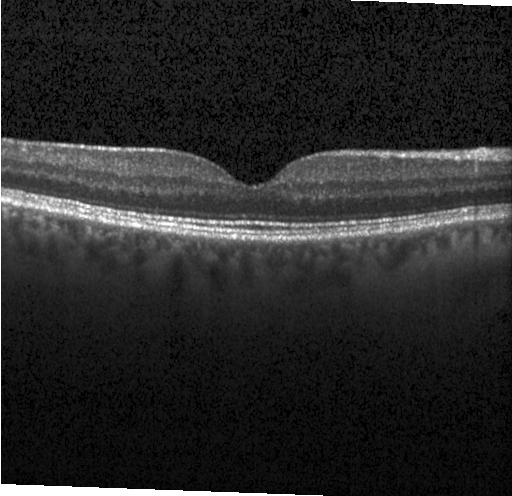

Optical coherence tomography B-scan.
Diagnosis: neither choroidal neovascularization, diabetic macular edema, nor drusen.